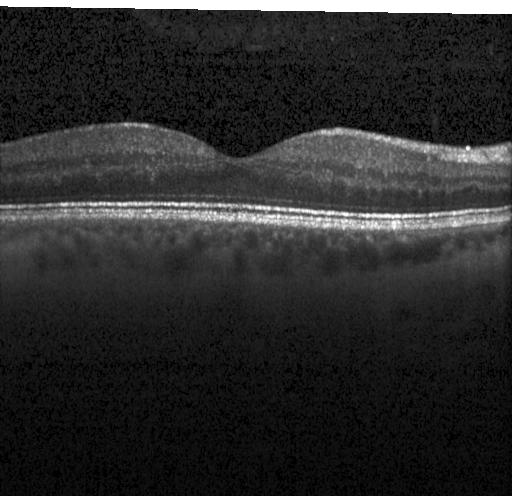

Optical coherence tomography scan · spectral-domain OCT — Impression: neither choroidal neovascularization, diabetic macular edema, nor drusen.